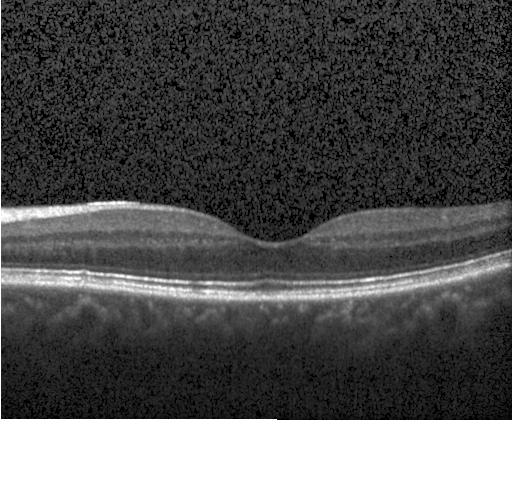 Impression: neither choroidal neovascularization, diabetic macular edema, nor drusen.